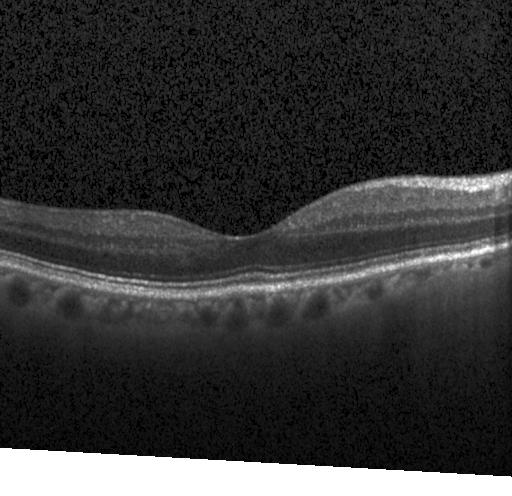 OCT scan showing no choroidal neovascularization, no diabetic macular edema, and no drusen.